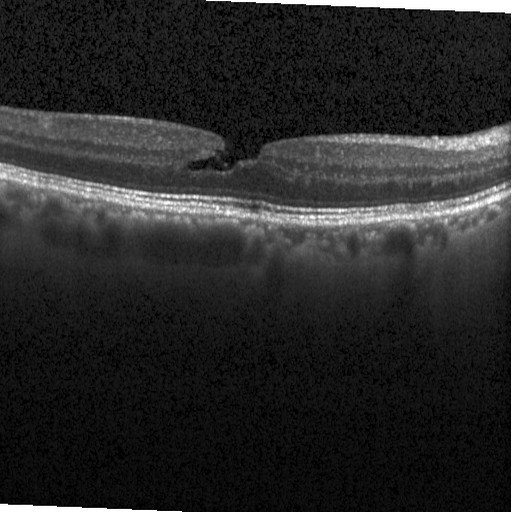

Spectral-domain optical coherence tomography · OCT B-scan · acquired on a Heidelberg Spectralis
The scan shows diabetic macular edema.